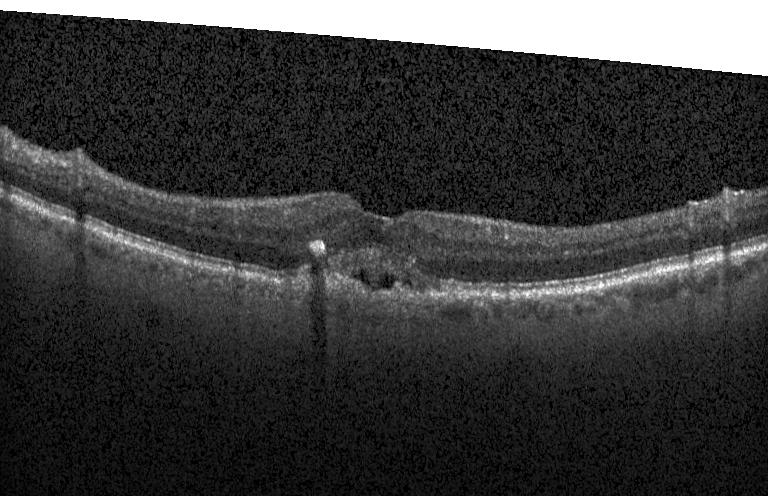

Spectral-domain optical coherence tomography · through the macula · OCT B-scan. Diagnosis: a choroidal neovascular membrane.